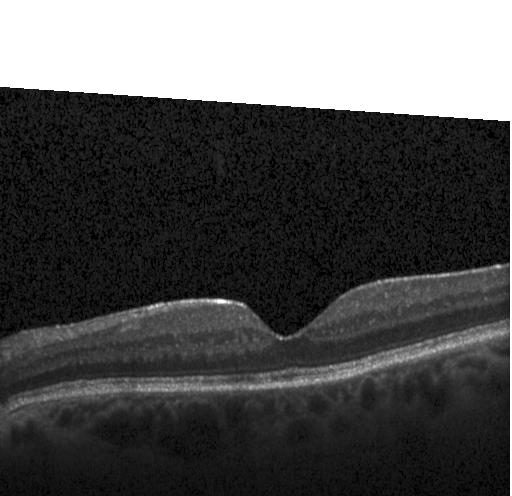
Heidelberg Spectralis; retinal OCT cross-section; spectral-domain OCT
No choroidal neovascularization, no diabetic macular edema, and no drusen.